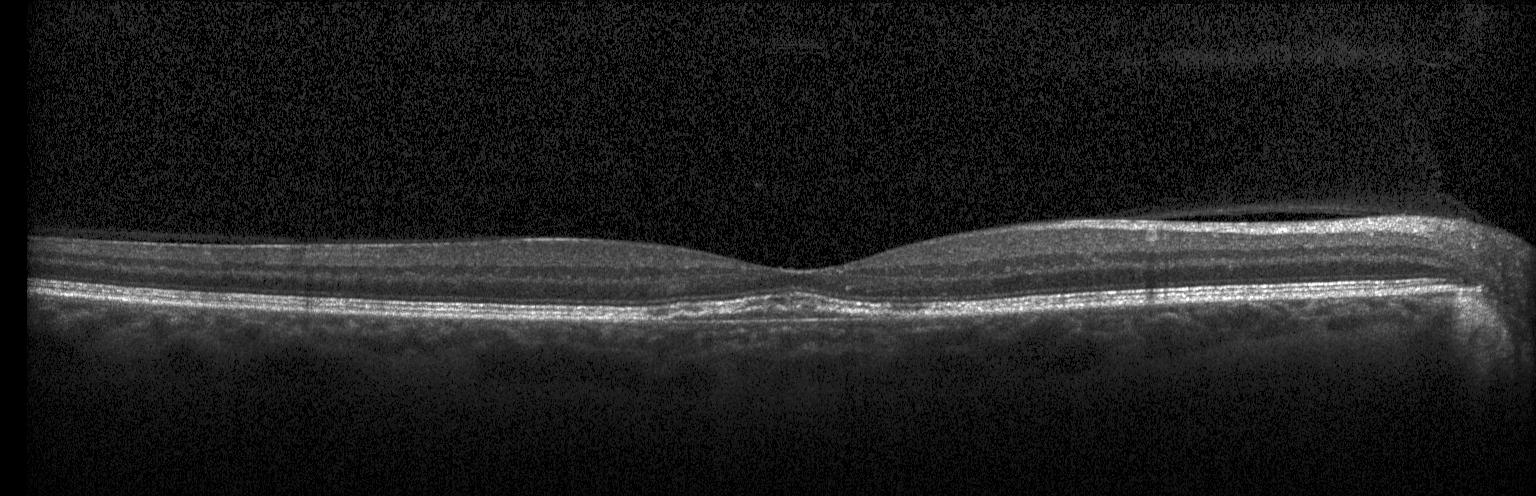 OCT B-scan showing a choroidal neovascular membrane.